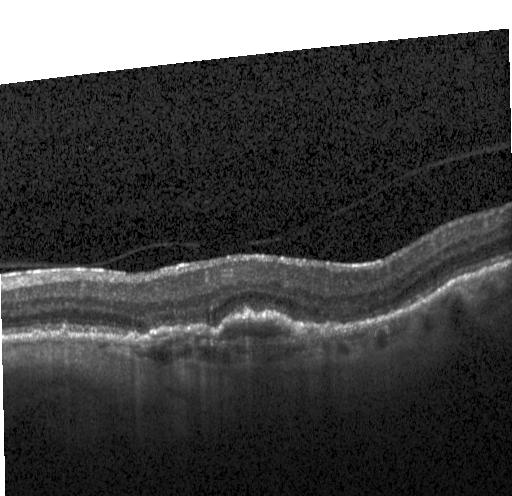 Spectral-domain OCT, acquired on a Heidelberg Spectralis, OCT line scan, horizontal scan through the fovea. Macular OCT: a choroidal neovascular membrane.